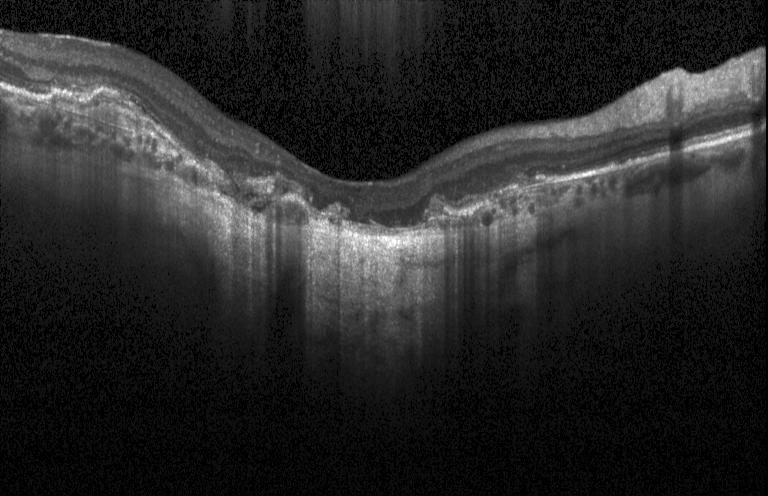
Retinal OCT cross-section, Heidelberg Spectralis, fovea-centered. A choroidal neovascular membrane.